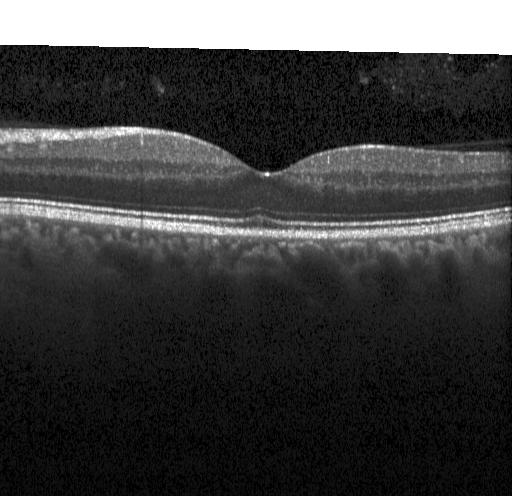
Optical coherence tomography B-scan — Diagnosis: no evidence of choroidal neovascularization, diabetic macular edema, or drusen.